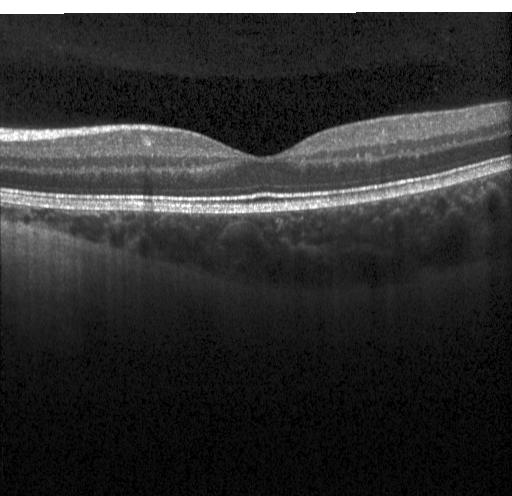 No evidence of CNV, DME, or drusen.